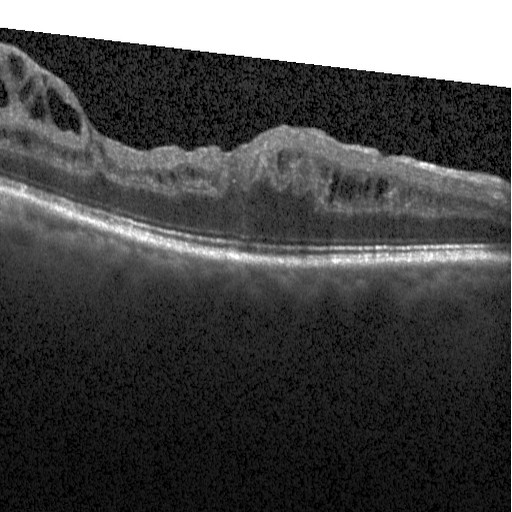

Impression: DME.